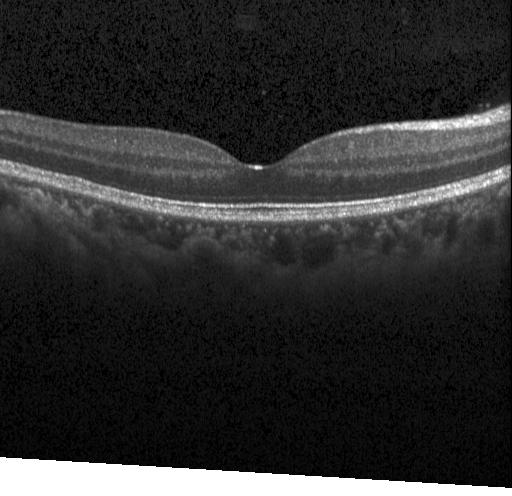

Optical coherence tomography scan. Heidelberg Spectralis. The scan shows no choroidal neovascularization, diabetic macular edema, or drusen.